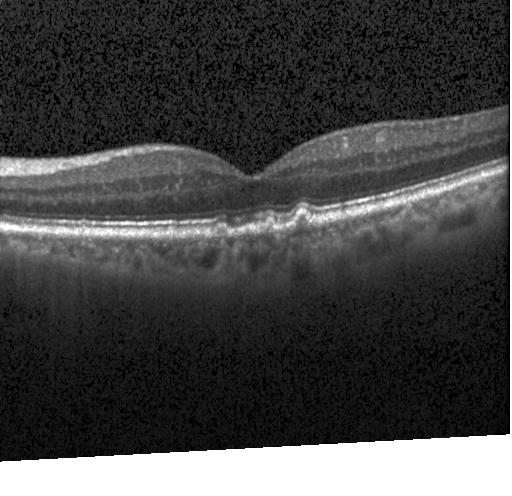
Centered on the fovea. Optical coherence tomography B-scan. Acquired on a Heidelberg Spectralis.
Diagnosis: drusen.